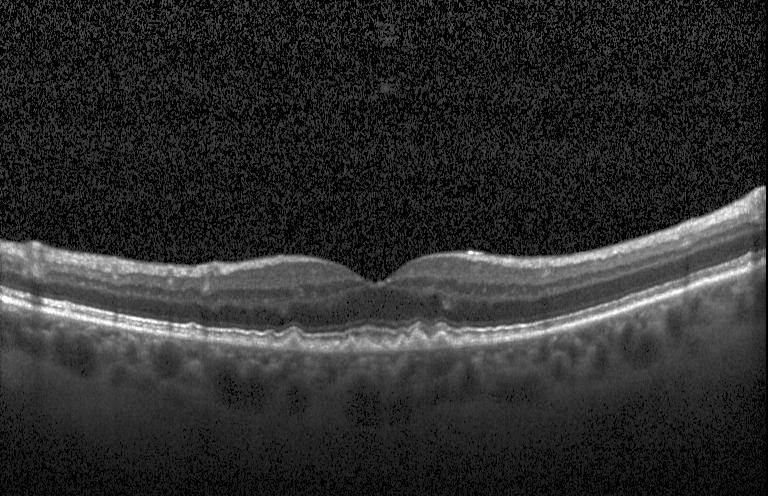 Optical coherence tomography B-scan.
Finding: drusen.